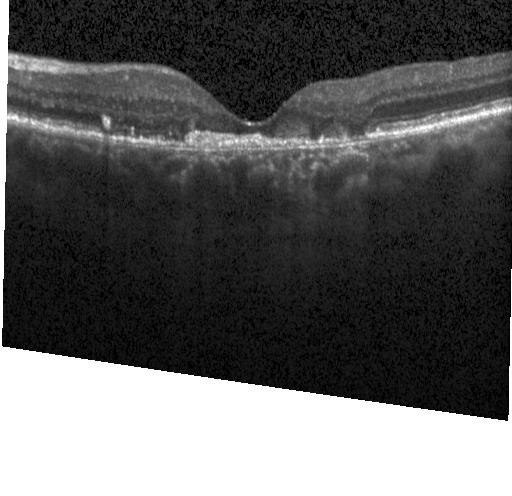

Spectral-domain OCT. Optical coherence tomography B-scan. Fovea-centered. Impression: CNV.